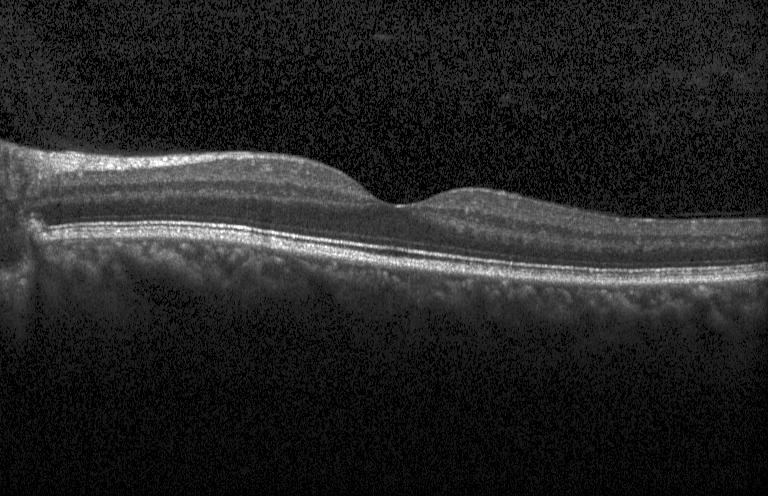 Dx: neither choroidal neovascularization, diabetic macular edema, nor drusen.